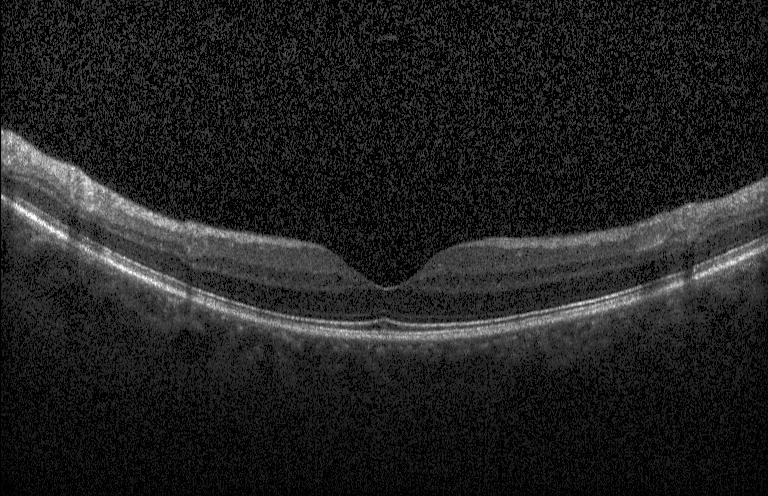
Finding: neither choroidal neovascularization, diabetic macular edema, nor drusen.